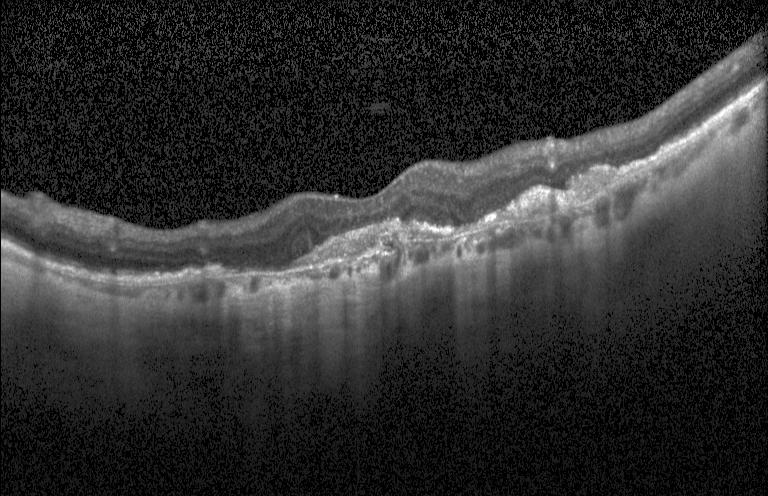 The scan shows a choroidal neovascular membrane.